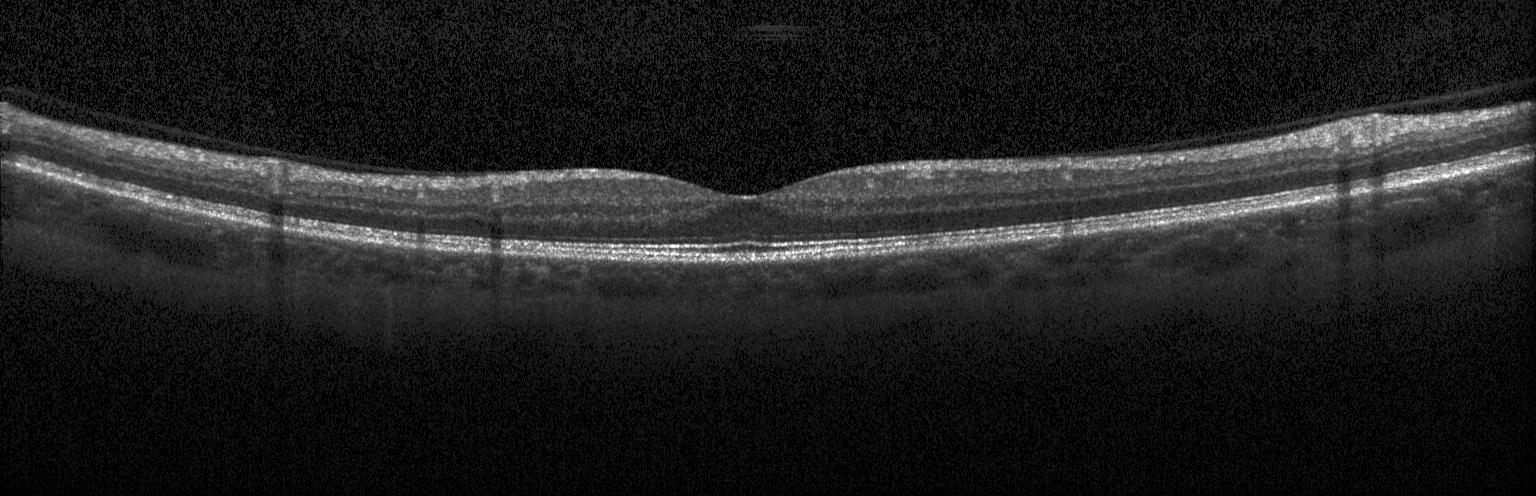
Retinal OCT cross-section showing no evidence of choroidal neovascularization, diabetic macular edema, or drusen.